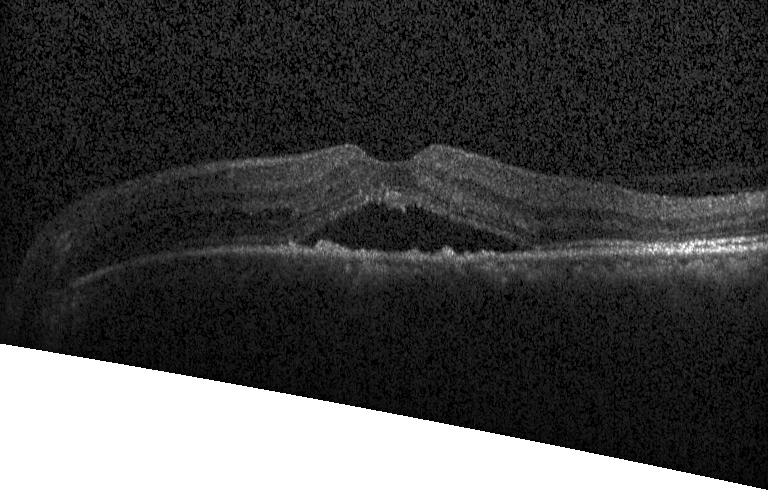 Optical coherence tomography B-scan, horizontal scan through the fovea — Impression: a choroidal neovascular membrane.